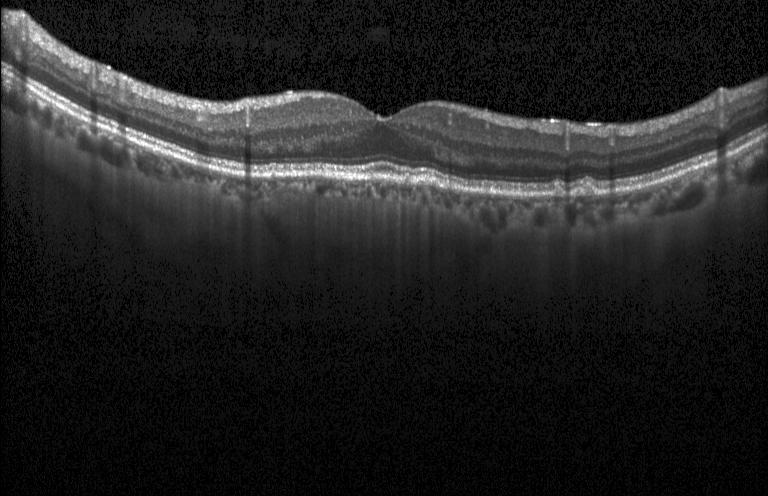

OCT B-scan, spectral-domain OCT, instrument: Heidelberg Spectralis. Macular OCT: sub-RPE drusenoid deposits.